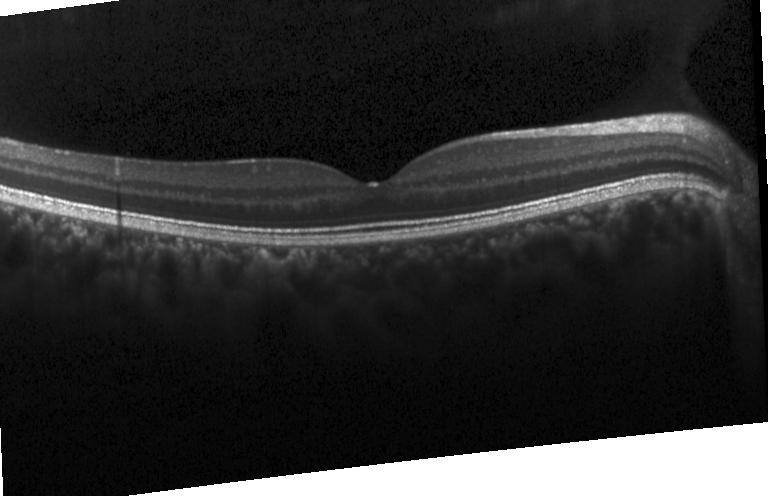

Instrument: Heidelberg Spectralis, optical coherence tomography B-scan, through the macula — Assessment: no CNV, no DME, and no drusen.